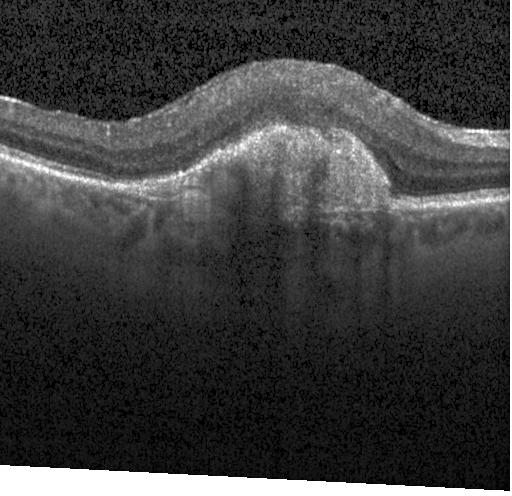
OCT finding: choroidal neovascularization (CNV).